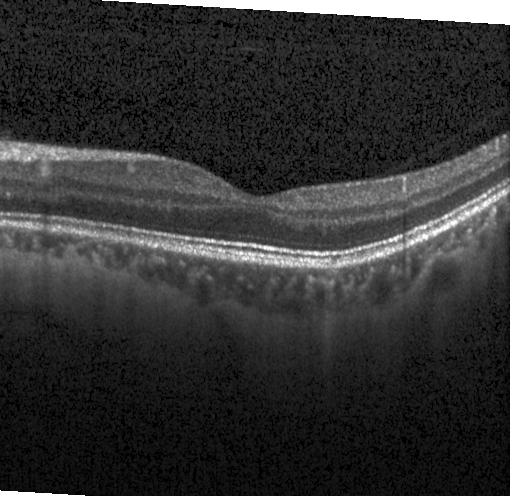
OCT line scan.
Diagnosis: no choroidal neovascularization, no diabetic macular edema, and no drusen.